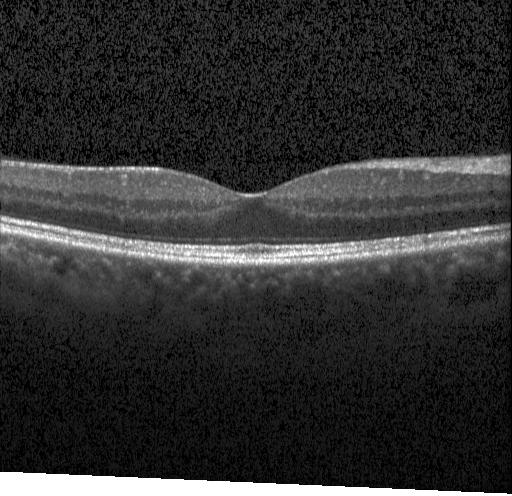 Finding: no evidence of choroidal neovascularization, diabetic macular edema, or drusen.